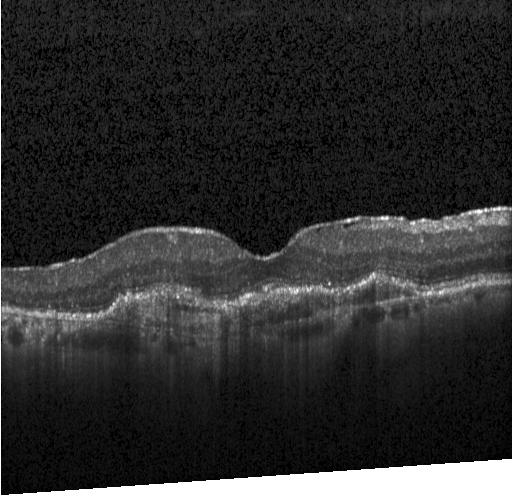
Diagnosis: a choroidal neovascular membrane.